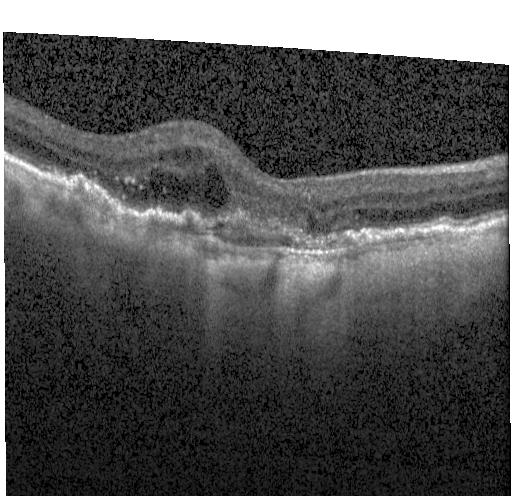
Dx: a choroidal neovascular membrane.